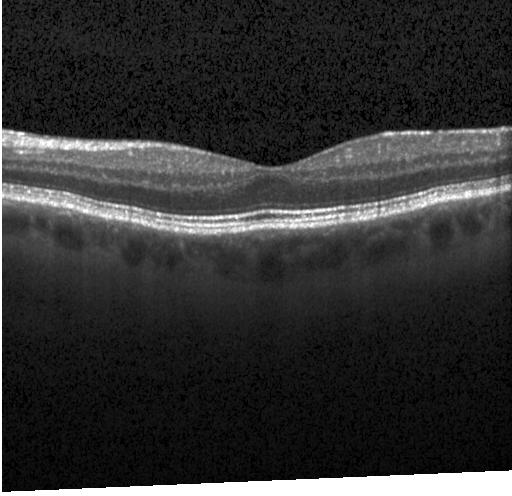

Macular scan; instrument: Heidelberg Spectralis; SD-OCT; retinal OCT B-scan. Macular OCT: neither choroidal neovascularization, diabetic macular edema, nor drusen.